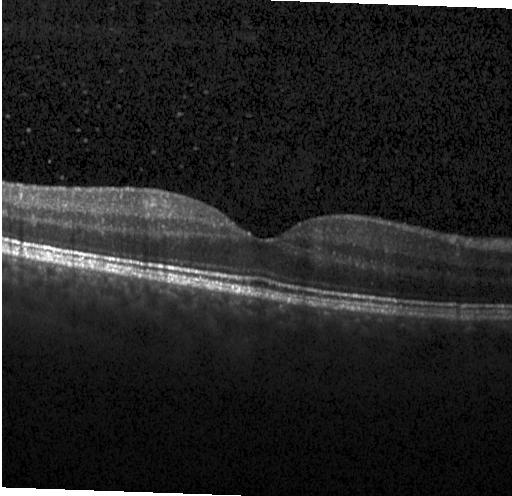

Macular scan; Heidelberg Spectralis OCT system; OCT B-scan. Finding: no evidence of choroidal neovascularization, diabetic macular edema, or drusen.